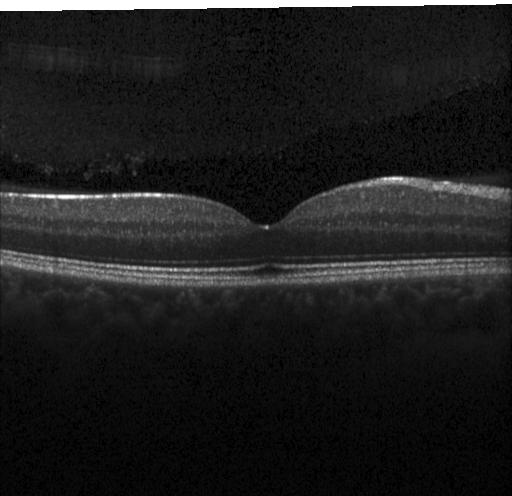 Retinal OCT cross-section, centered on the fovea, Heidelberg Spectralis, SD-OCT — Finding: no choroidal neovascularization, no diabetic macular edema, and no drusen.